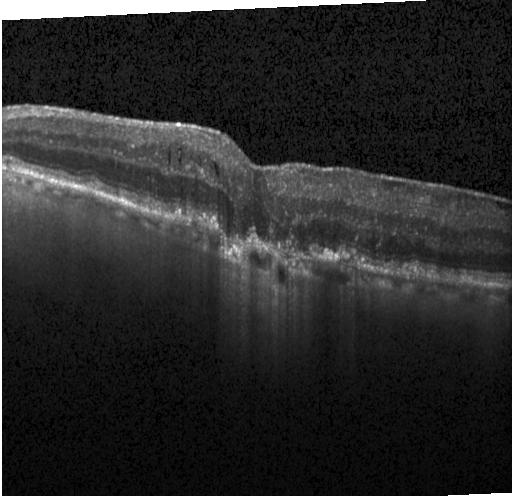

Assessment: a choroidal neovascular membrane.